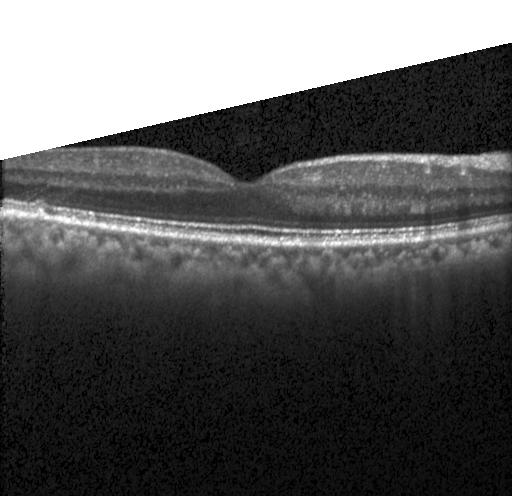

Optical coherence tomography B-scan.
This B-scan demonstrates neither choroidal neovascularization, diabetic macular edema, nor drusen.